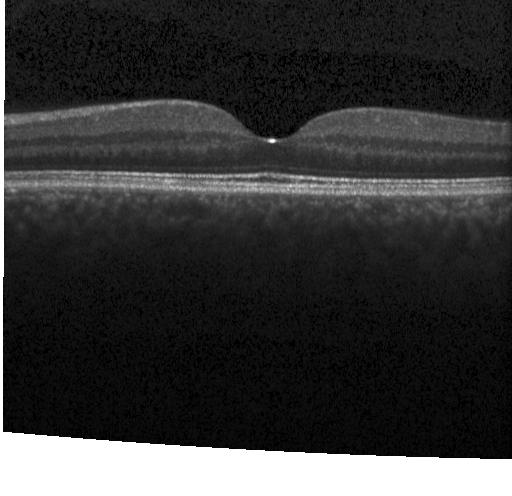 OCT line scan
Finding: no choroidal neovascularization, no diabetic macular edema, and no drusen.